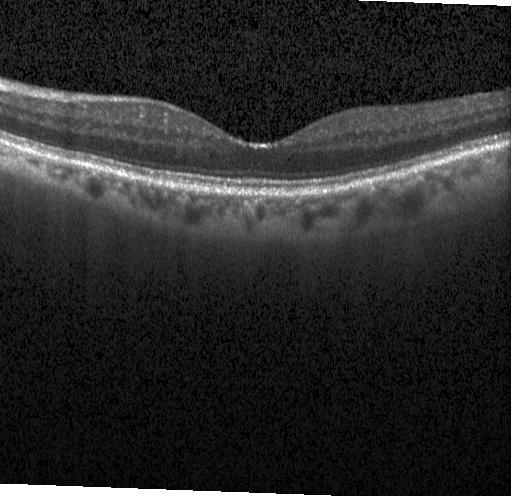 Instrument: Heidelberg Spectralis · optical coherence tomography B-scan · spectral-domain optical coherence tomography. Dx: no choroidal neovascularization, diabetic macular edema, or drusen.